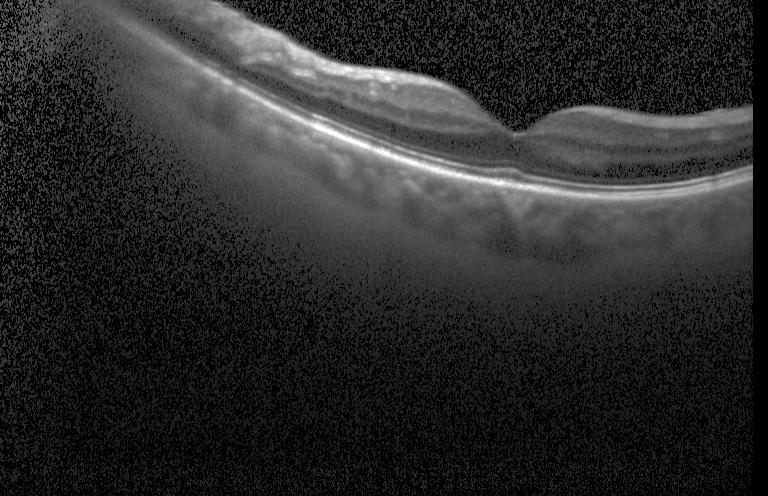

SD-OCT. Retinal OCT B-scan. Acquired on a Heidelberg Spectralis.
Impression: no evidence of CNV, DME, or drusen.